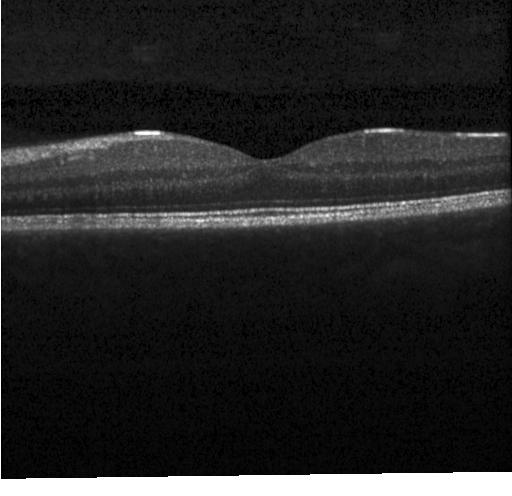
Dx: no choroidal neovascularization, diabetic macular edema, or drusen.